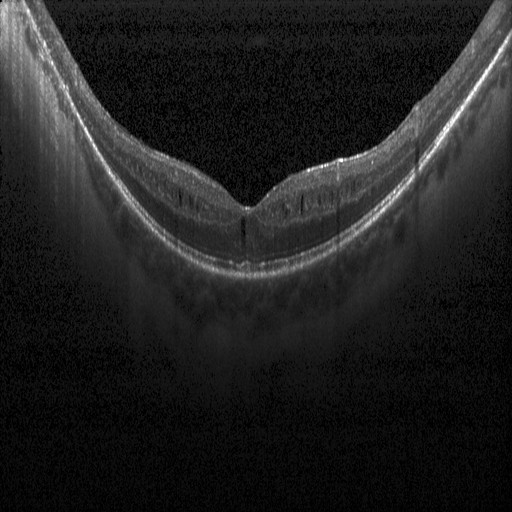
Heidelberg Spectralis OCT system, OCT B-scan, centered on the fovea
Impression: diabetic macular edema (DME).